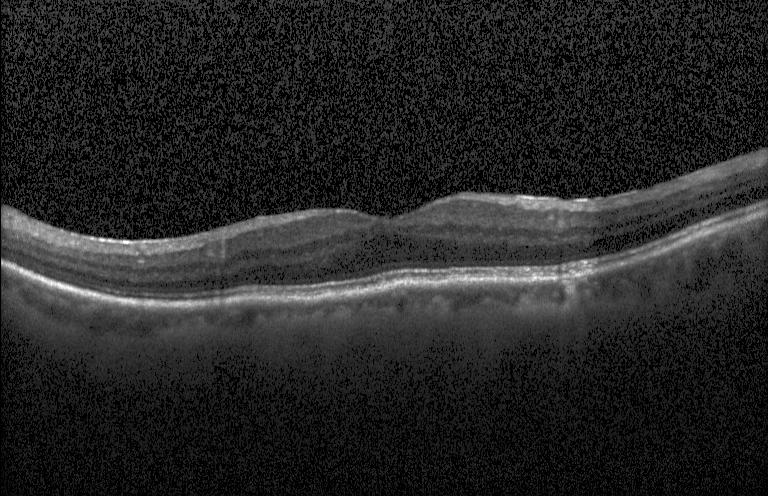

Macular OCT: no choroidal neovascularization, no diabetic macular edema, and no drusen.